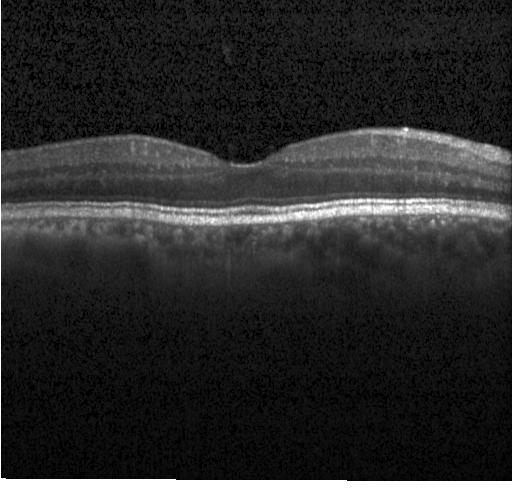

Instrument: Heidelberg Spectralis. OCT B-scan. Diagnosis: no evidence of CNV, DME, or drusen.